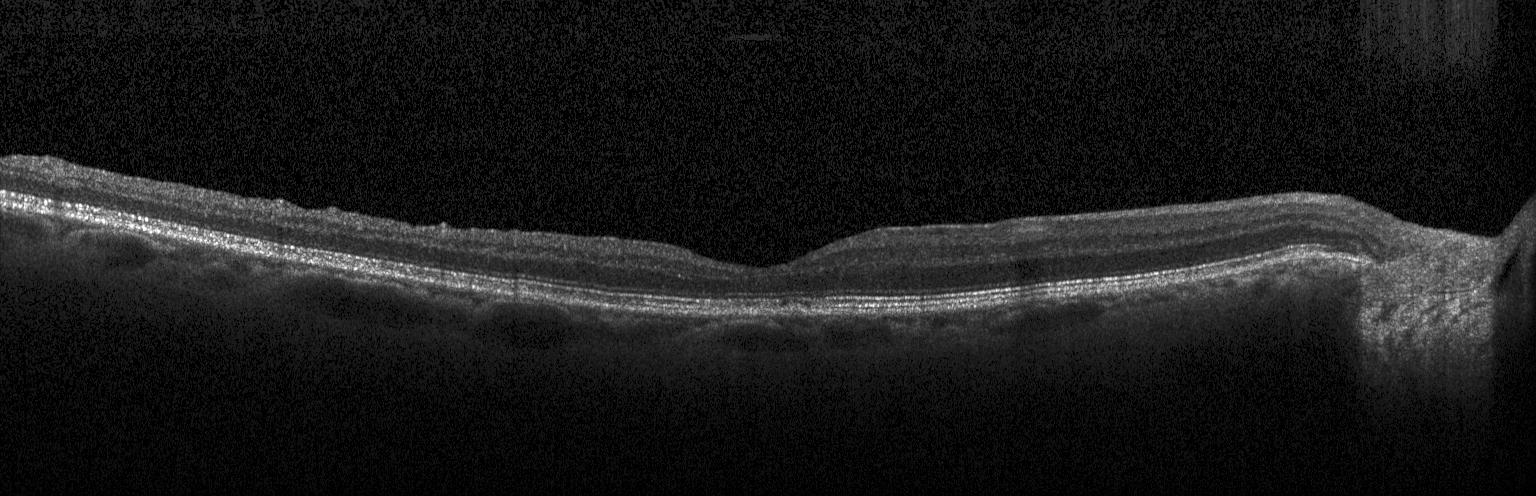 Heidelberg Spectralis. Optical coherence tomography B-scan. Macular scan. SD-OCT. Impression: no evidence of choroidal neovascularization, diabetic macular edema, or drusen.